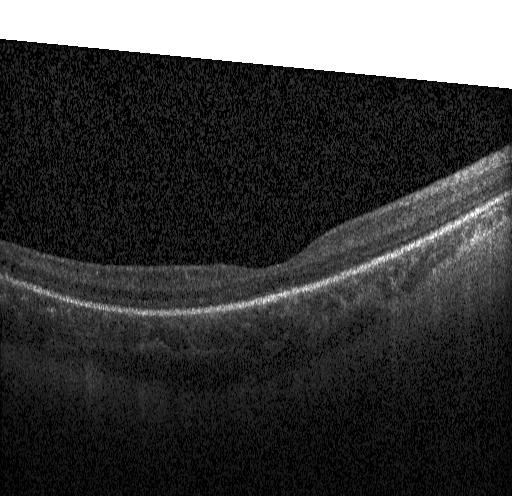 OCT line scan. Heidelberg Spectralis OCT system. Macular scan — Impression: no evidence of choroidal neovascularization, diabetic macular edema, or drusen.